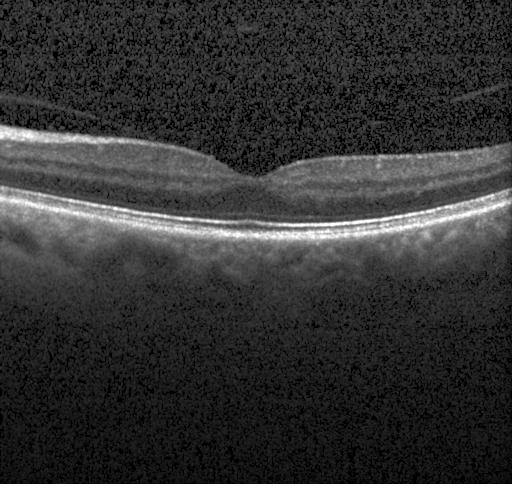
Heidelberg Spectralis. Retinal OCT B-scan
Diagnosis: no choroidal neovascularization, diabetic macular edema, or drusen.